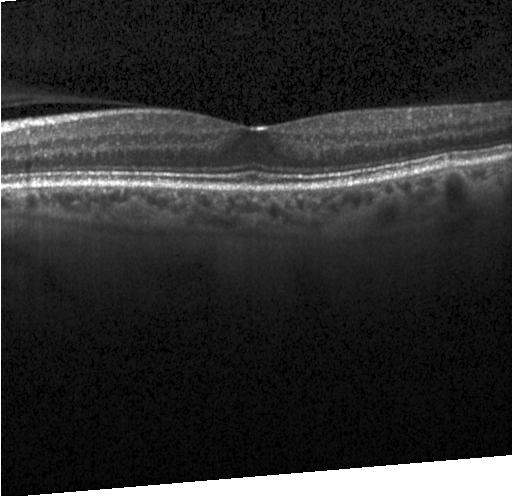
Centered on the fovea, OCT line scan — Diagnosis: neither choroidal neovascularization, diabetic macular edema, nor drusen.